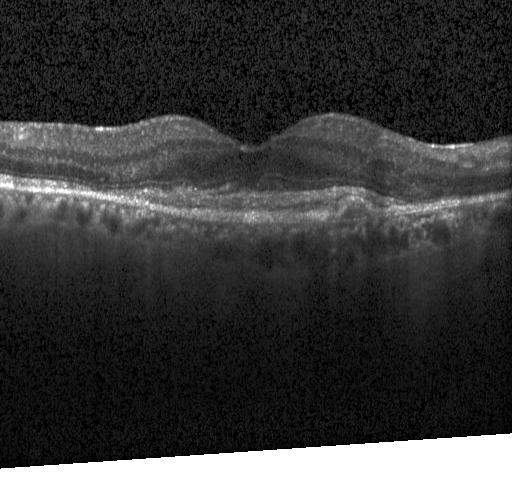
OCT B-scan showing a choroidal neovascular membrane.